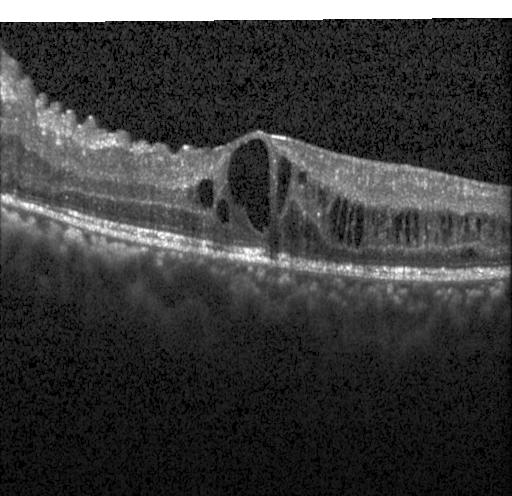

Spectral-domain OCT, retinal OCT B-scan.
Finding: DME.